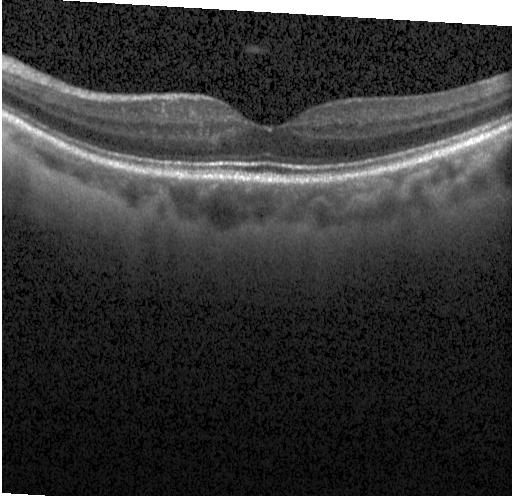

Impression: no evidence of CNV, DME, or drusen.